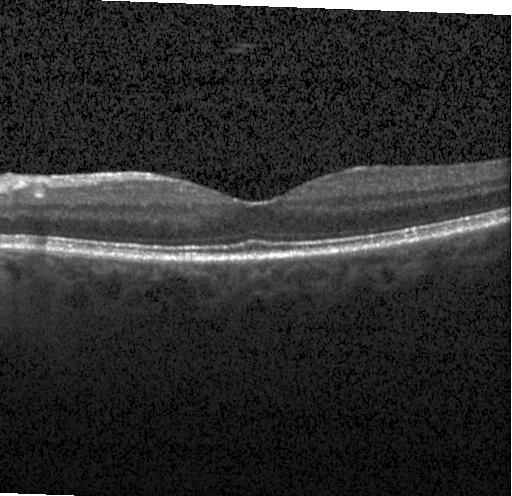

Optical coherence tomography scan; instrument: Heidelberg Spectralis; spectral-domain optical coherence tomography
Dx: no evidence of choroidal neovascularization, diabetic macular edema, or drusen.